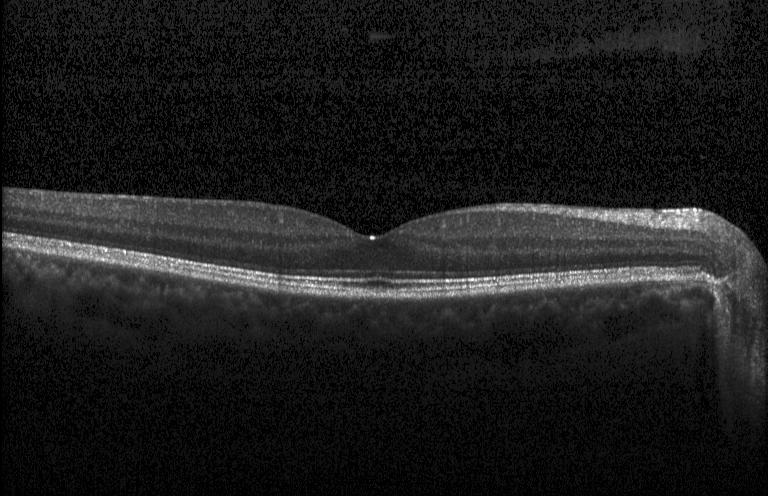

Optical coherence tomography B-scan. Macular scan. Spectral-domain OCT.
This B-scan demonstrates neither CNV, DME, nor drusen.